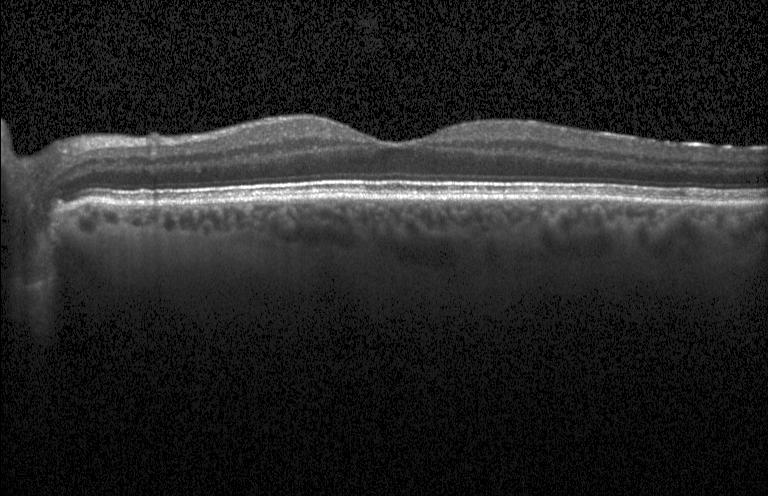

OCT line scan, through the macula. OCT finding: no evidence of choroidal neovascularization, diabetic macular edema, or drusen.